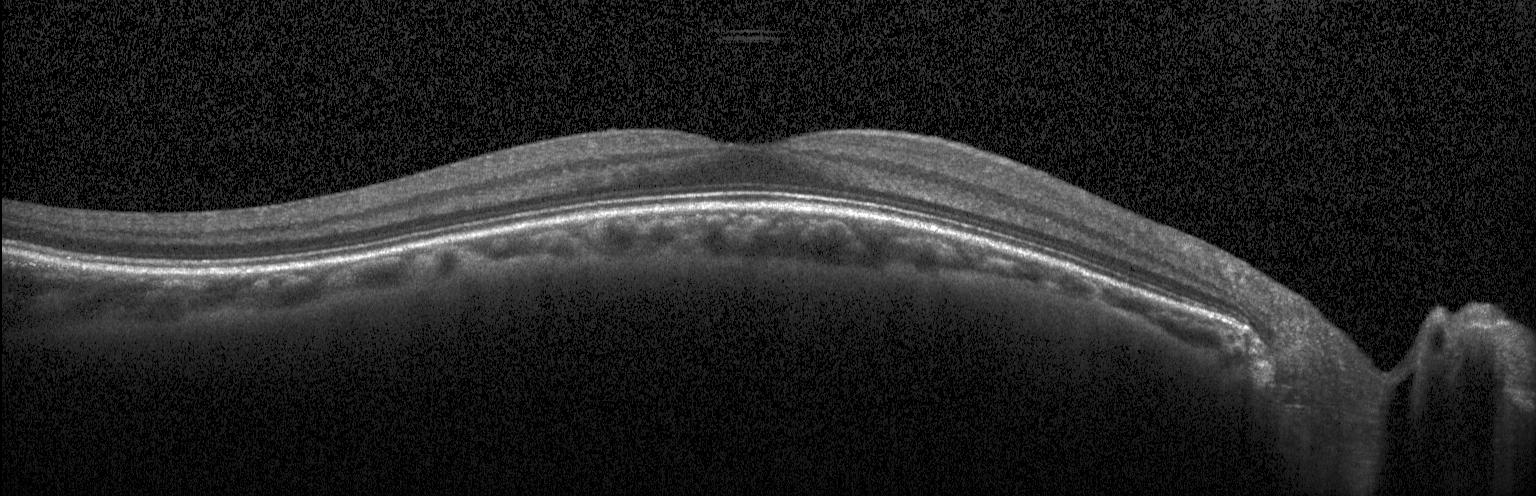

OCT B-scan showing no evidence of choroidal neovascularization, diabetic macular edema, or drusen.